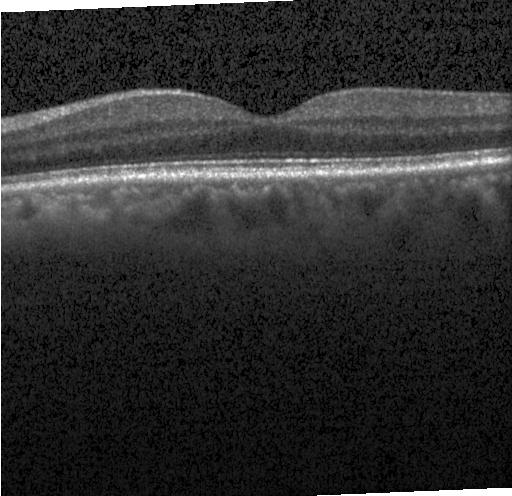 Finding: neither CNV, DME, nor drusen.